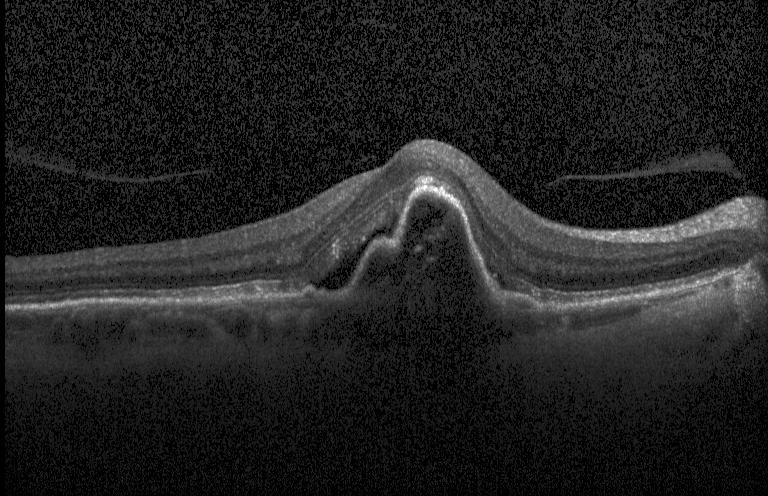
Spectral-domain optical coherence tomography; instrument: Heidelberg Spectralis; macular scan; optical coherence tomography scan. The scan shows a choroidal neovascular membrane.